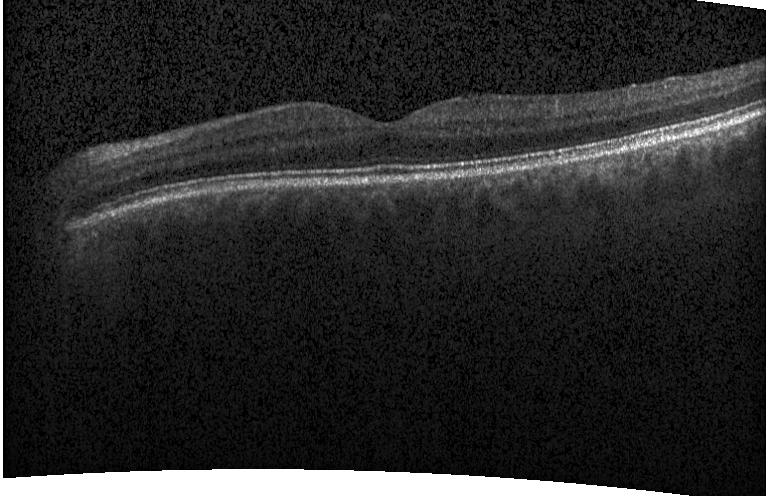 Heidelberg Spectralis OCT system; optical coherence tomography scan. This B-scan demonstrates no choroidal neovascularization, diabetic macular edema, or drusen.